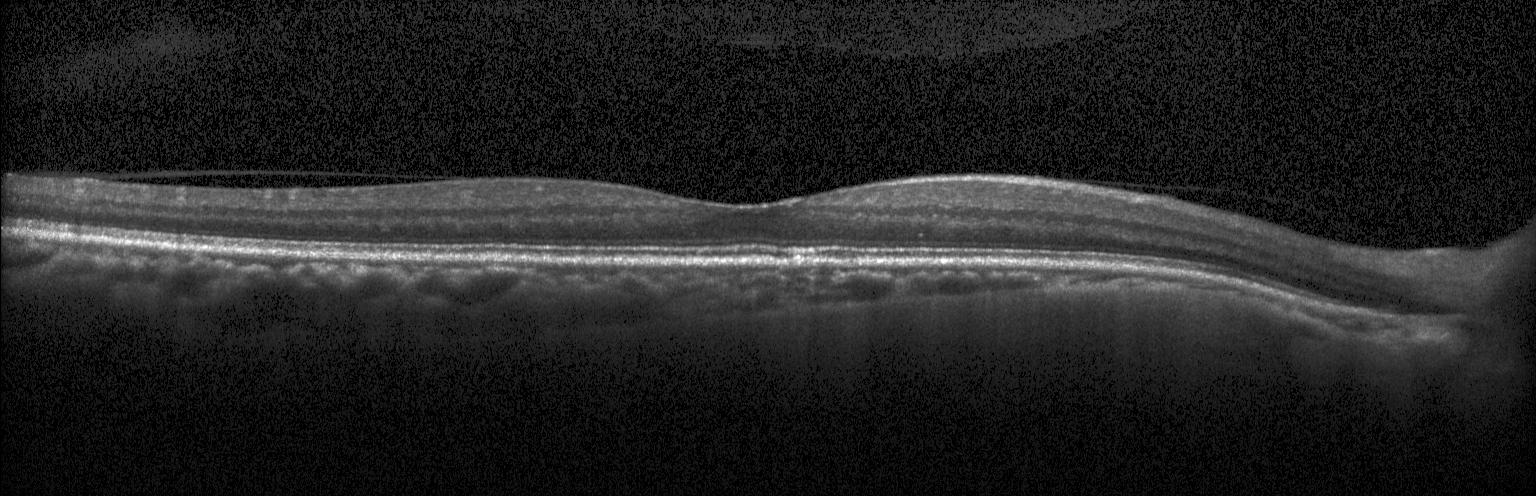
Retinal OCT cross-section
No evidence of CNV, DME, or drusen.